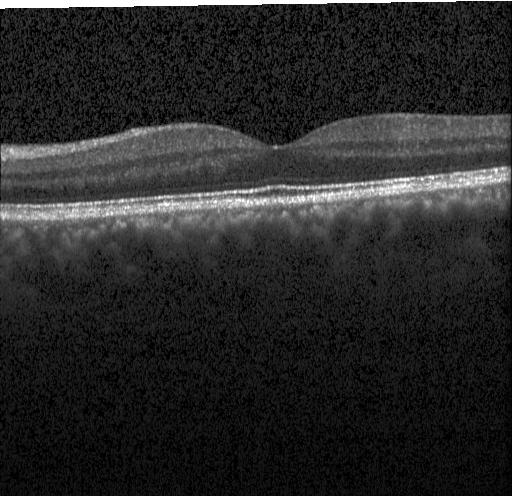
Optical coherence tomography B-scan
The scan shows neither choroidal neovascularization, diabetic macular edema, nor drusen.